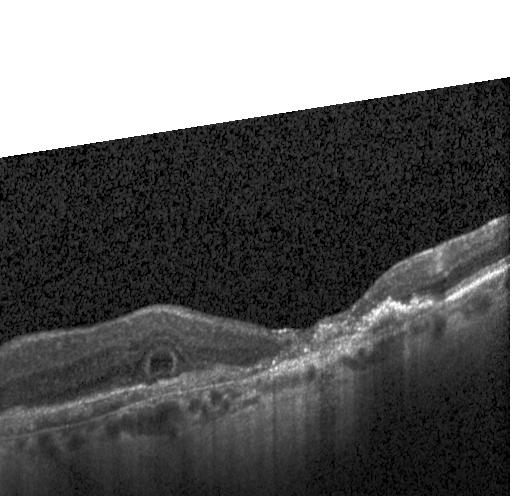 Optical coherence tomography scan, spectral-domain optical coherence tomography.
Dx: choroidal neovascularization.